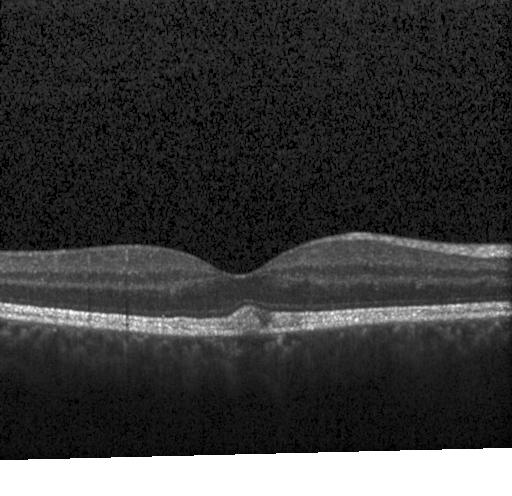
SD-OCT · OCT B-scan — Finding: sub-RPE drusenoid deposits.